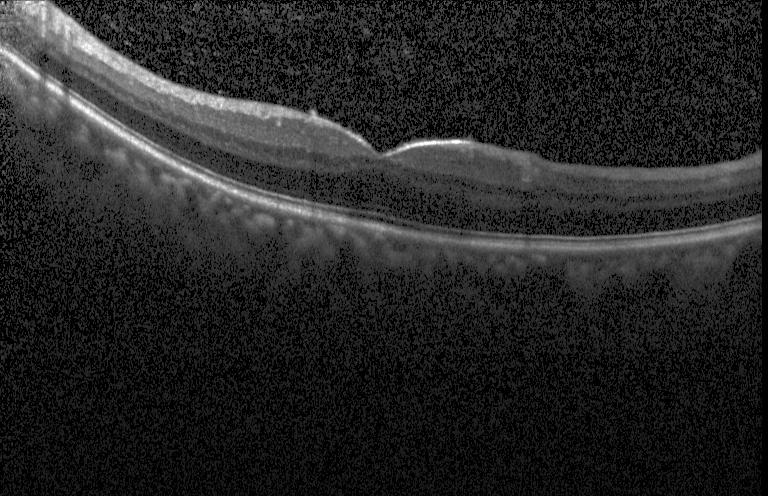
OCT scan showing no choroidal neovascularization, diabetic macular edema, or drusen.